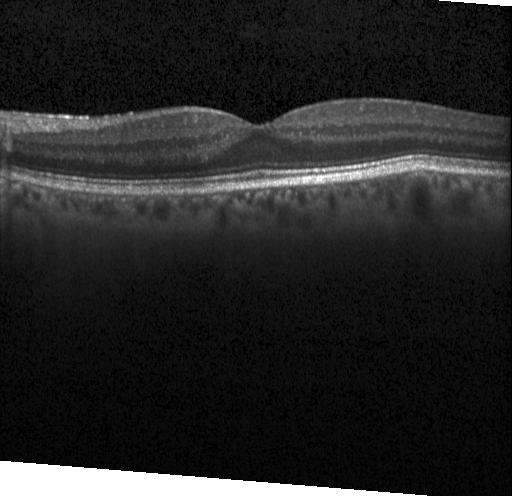

This B-scan demonstrates no choroidal neovascularization, diabetic macular edema, or drusen.